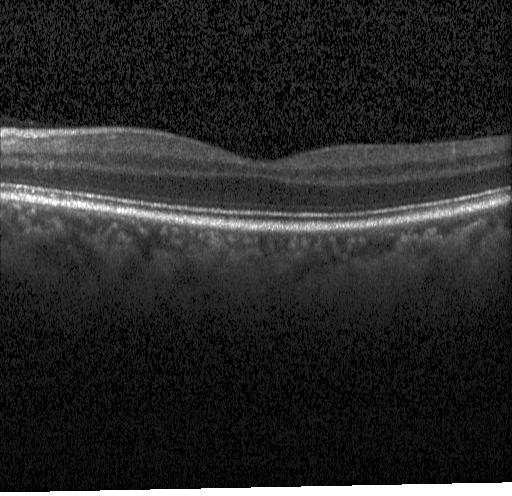
Spectral-domain OCT, OCT line scan, centered on the fovea. Diagnosis: neither choroidal neovascularization, diabetic macular edema, nor drusen.